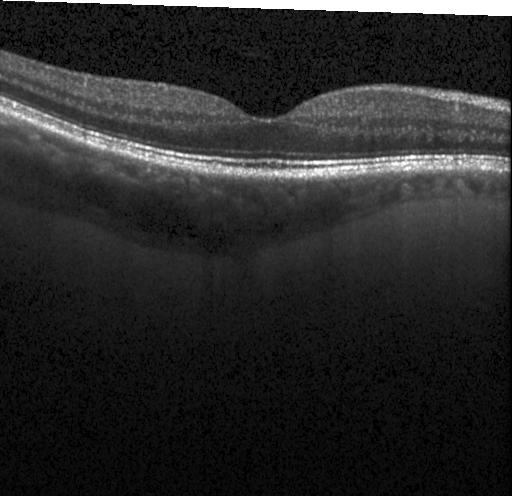

Finding: no choroidal neovascularization, diabetic macular edema, or drusen.